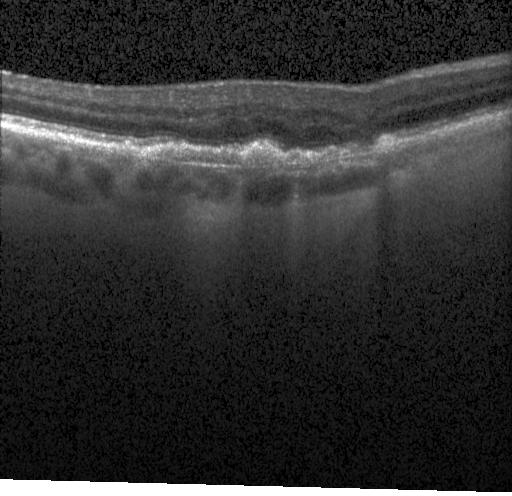
Macular OCT demonstrating a choroidal neovascular membrane.